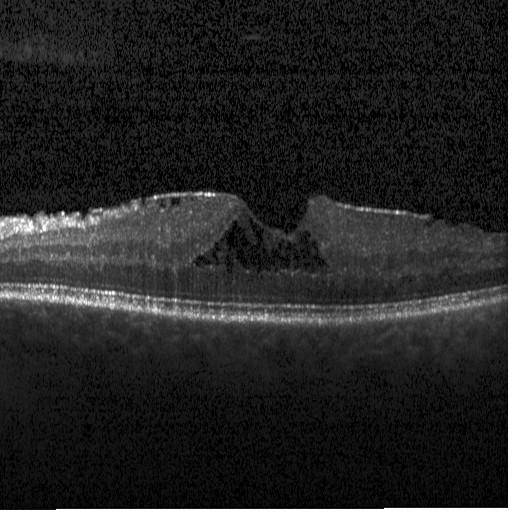
Retinal OCT cross-section showing diabetic macular edema (DME).